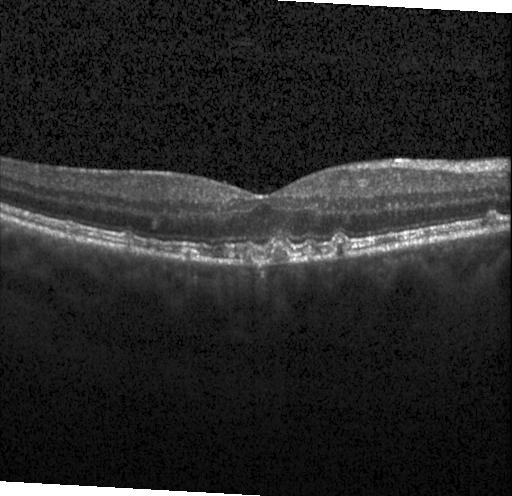
Impression: sub-RPE drusenoid deposits.